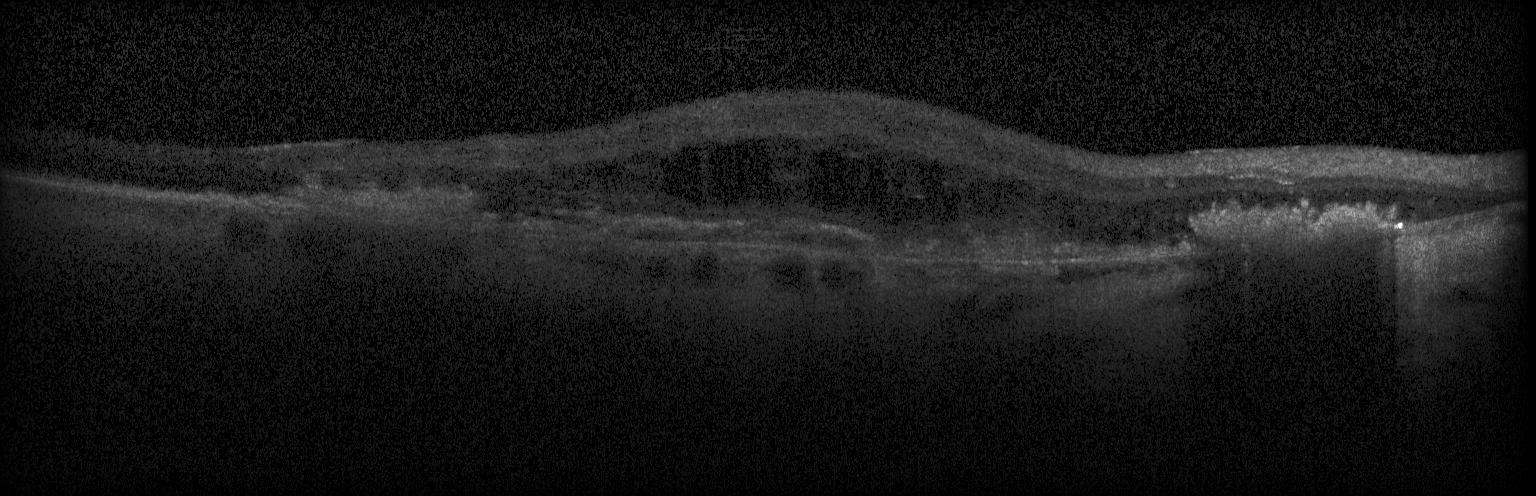 SD-OCT. OCT line scan. Centered on the fovea. Heidelberg Spectralis OCT system. Assessment: choroidal neovascularization (CNV).